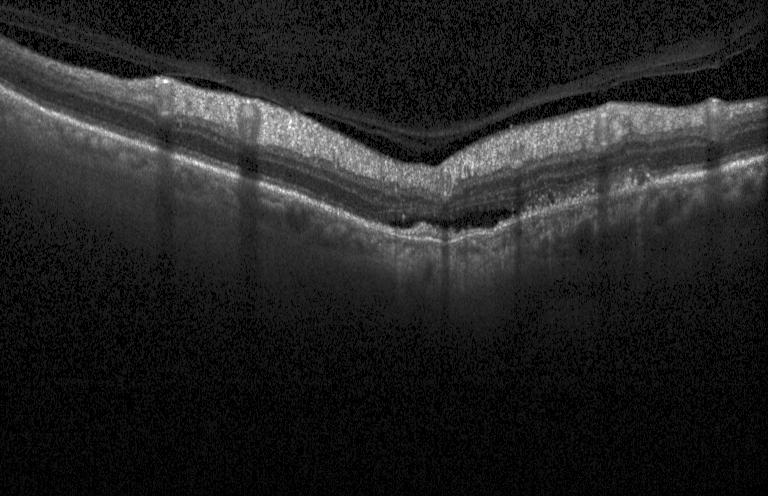

Impression: choroidal neovascularization (CNV).